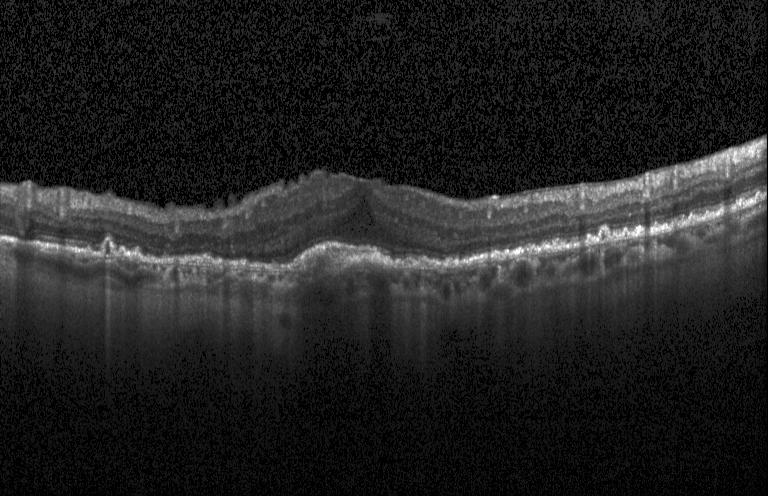 Finding: a choroidal neovascular membrane.